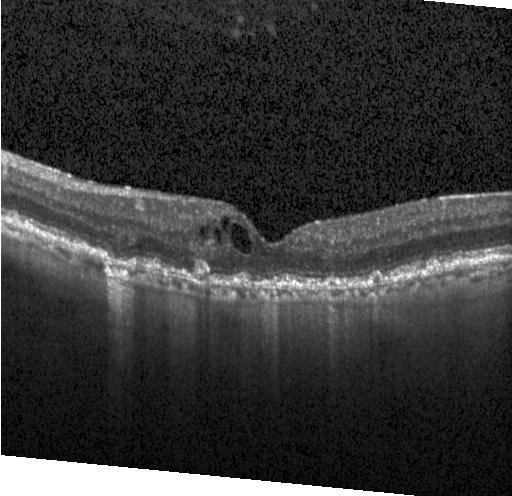
OCT scan showing a choroidal neovascular membrane.